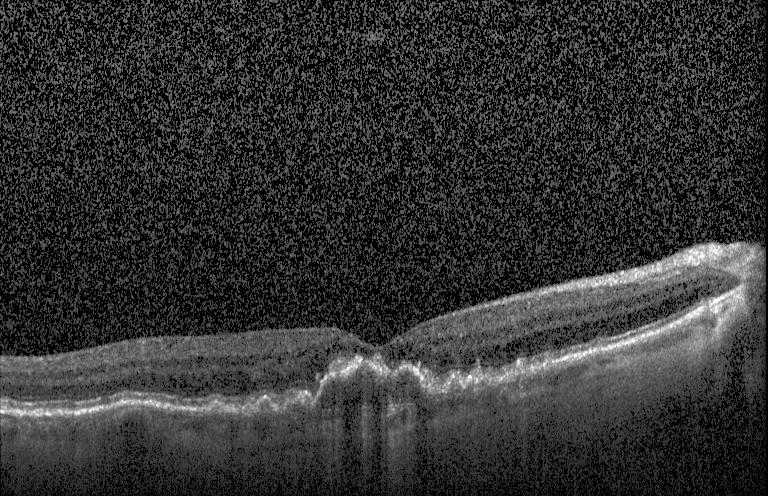

The scan shows a choroidal neovascular membrane.